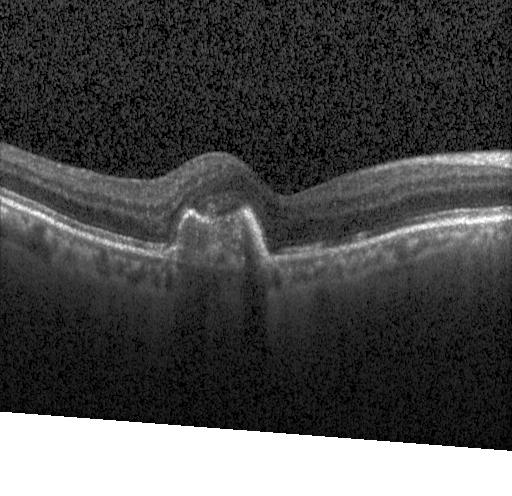 Macular OCT: a choroidal neovascular membrane.